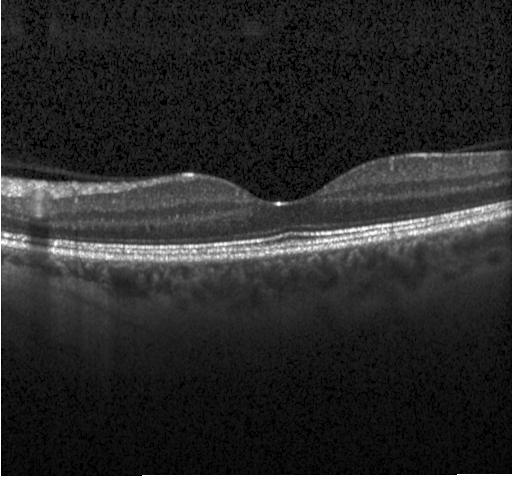

Diagnosis: no evidence of CNV, DME, or drusen.